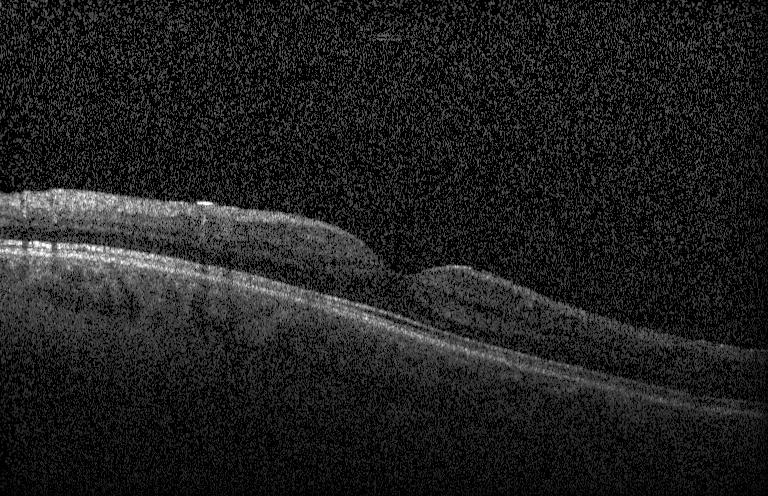 Spectral-domain optical coherence tomography, retinal OCT B-scan, instrument: Heidelberg Spectralis, through the macula. Finding: no CNV, DME, or drusen.